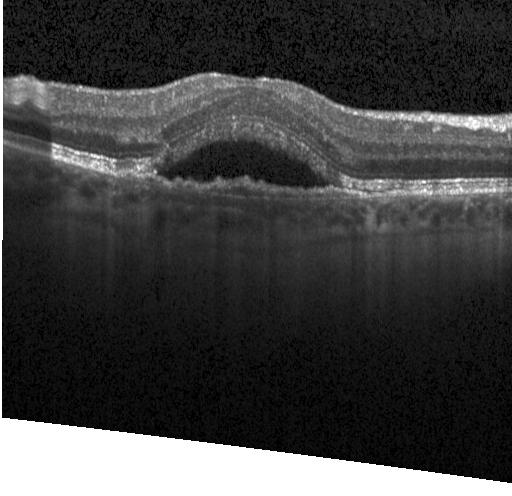 Spectral-domain OCT; optical coherence tomography scan; fovea-centered
Assessment: a choroidal neovascular membrane.